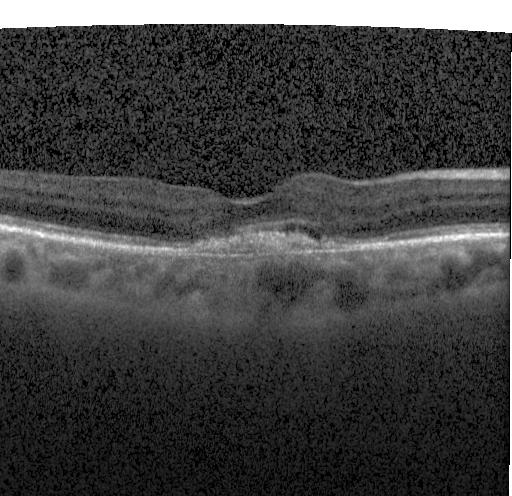

Acquired on a Heidelberg Spectralis · optical coherence tomography scan · fovea-centered · SD-OCT. Assessment: choroidal neovascularization (CNV).